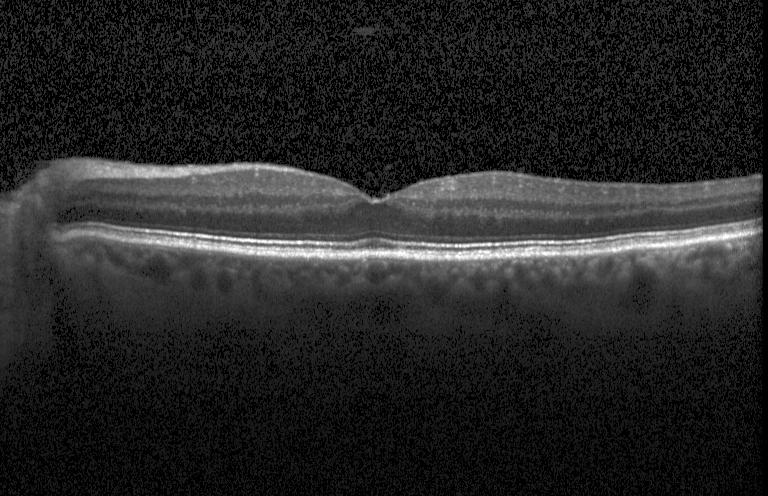

Retinal OCT cross-section. Horizontal scan through the fovea. Spectral-domain optical coherence tomography — Dx: no choroidal neovascularization, no diabetic macular edema, and no drusen.